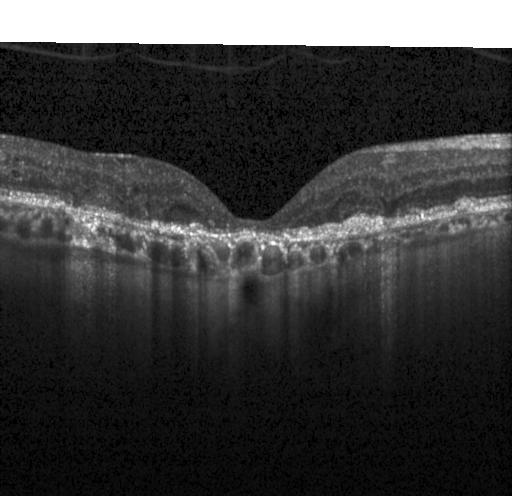
Retinal OCT cross-section. Acquired on a Heidelberg Spectralis. Spectral-domain optical coherence tomography
The scan shows a choroidal neovascular membrane.